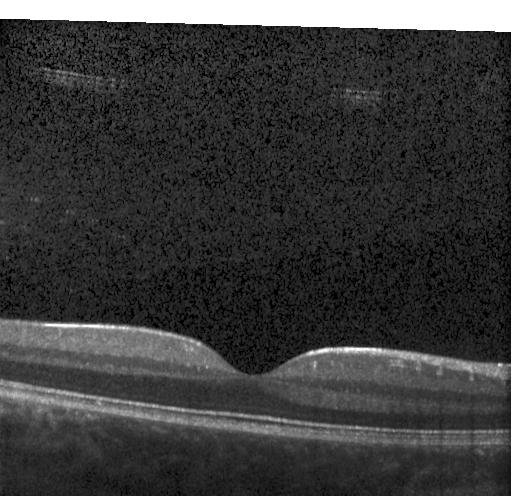 Optical coherence tomography scan.
OCT finding: no evidence of choroidal neovascularization, diabetic macular edema, or drusen.